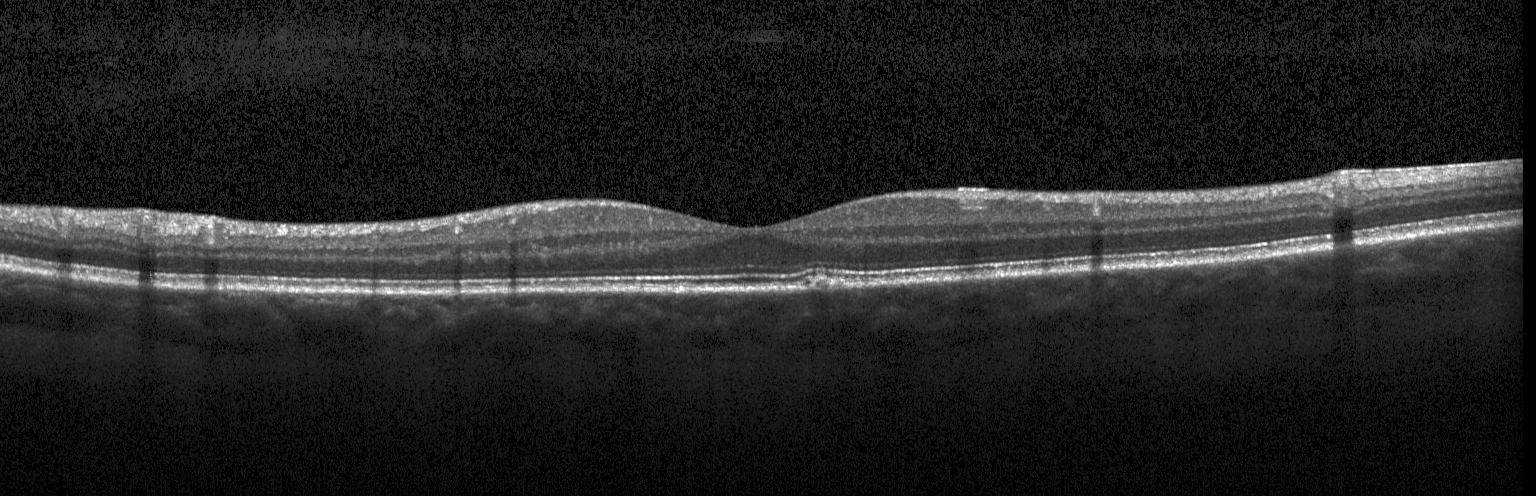 The scan shows multiple drusen.